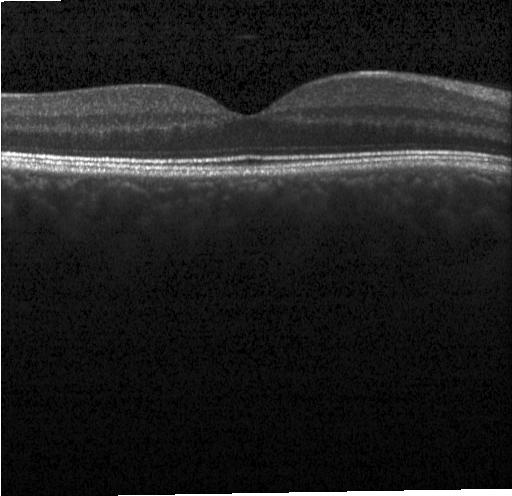 Macular scan. Retinal OCT B-scan
Diagnosis: no choroidal neovascularization, diabetic macular edema, or drusen.